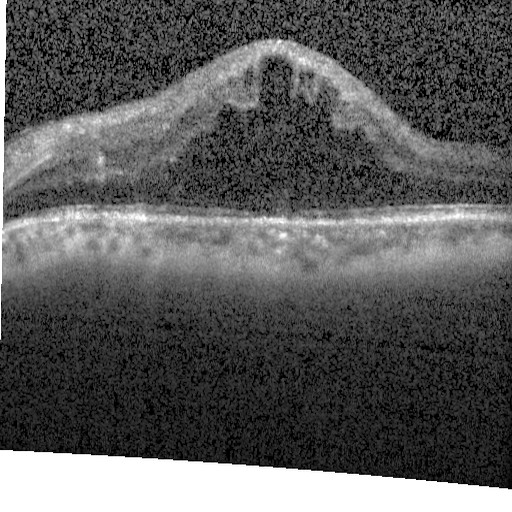

Through the macula, spectral-domain OCT, optical coherence tomography scan
OCT finding: diabetic macular edema.